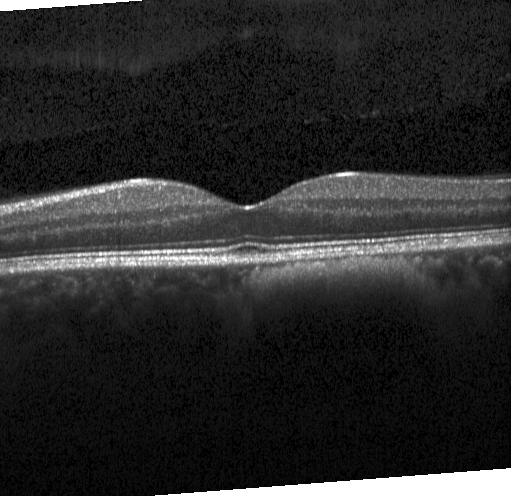

OCT B-scan showing no choroidal neovascularization, no diabetic macular edema, and no drusen.